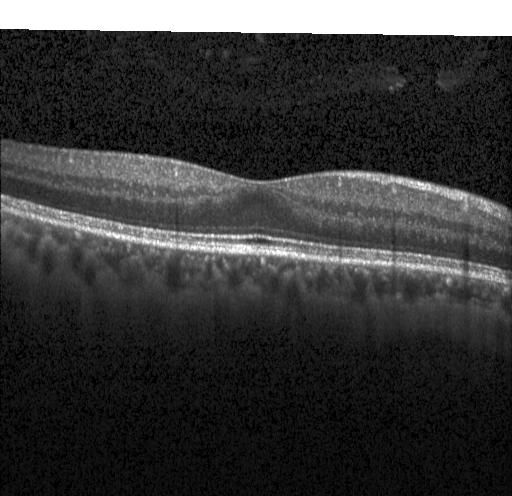

Retinal OCT cross-section — Impression: no choroidal neovascularization, diabetic macular edema, or drusen.